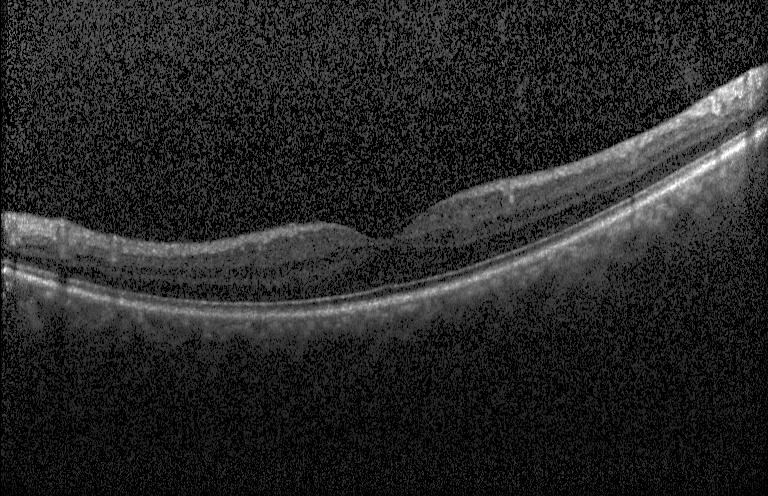 OCT line scan · instrument: Heidelberg Spectralis. No choroidal neovascularization, no diabetic macular edema, and no drusen.